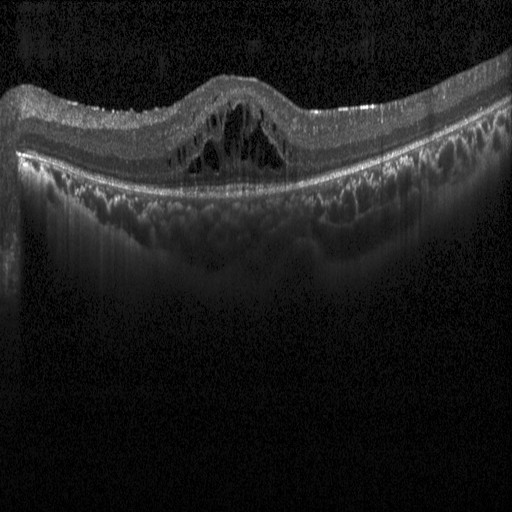
Macular OCT: diabetic macular edema (DME).